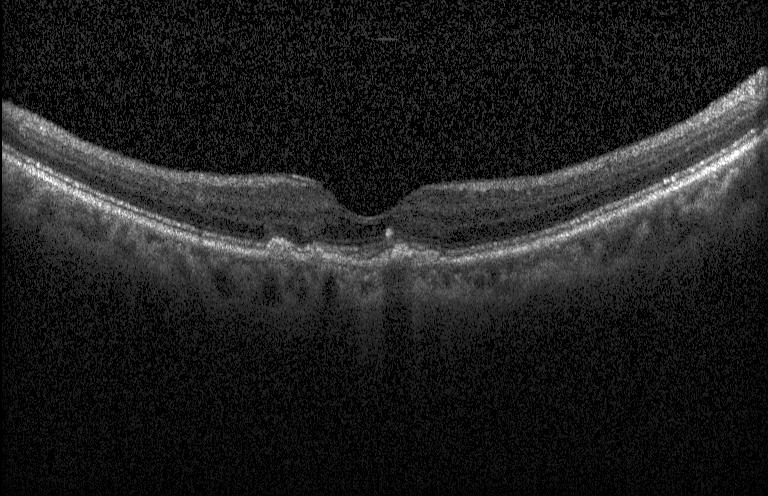

Diagnosis: a choroidal neovascular membrane.